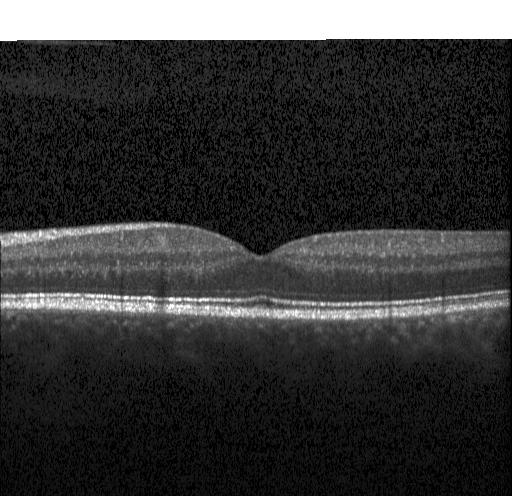 OCT line scan — Finding: neither CNV, DME, nor drusen.